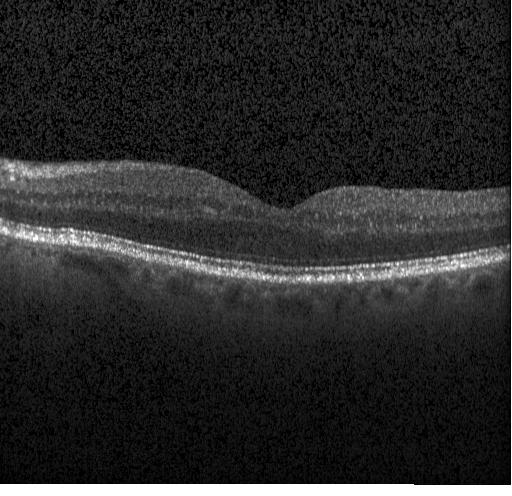 OCT scan showing no evidence of choroidal neovascularization, diabetic macular edema, or drusen.